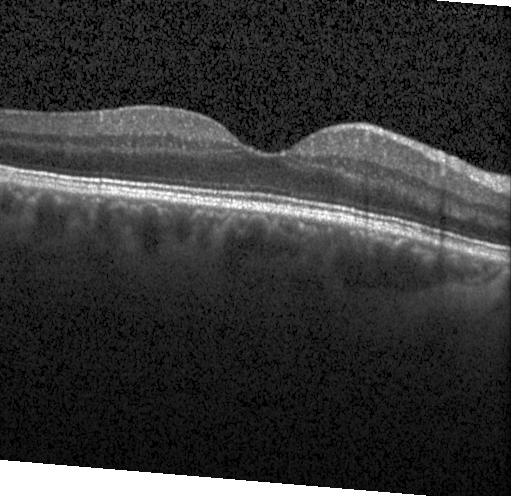

Macular OCT: no choroidal neovascularization, diabetic macular edema, or drusen.